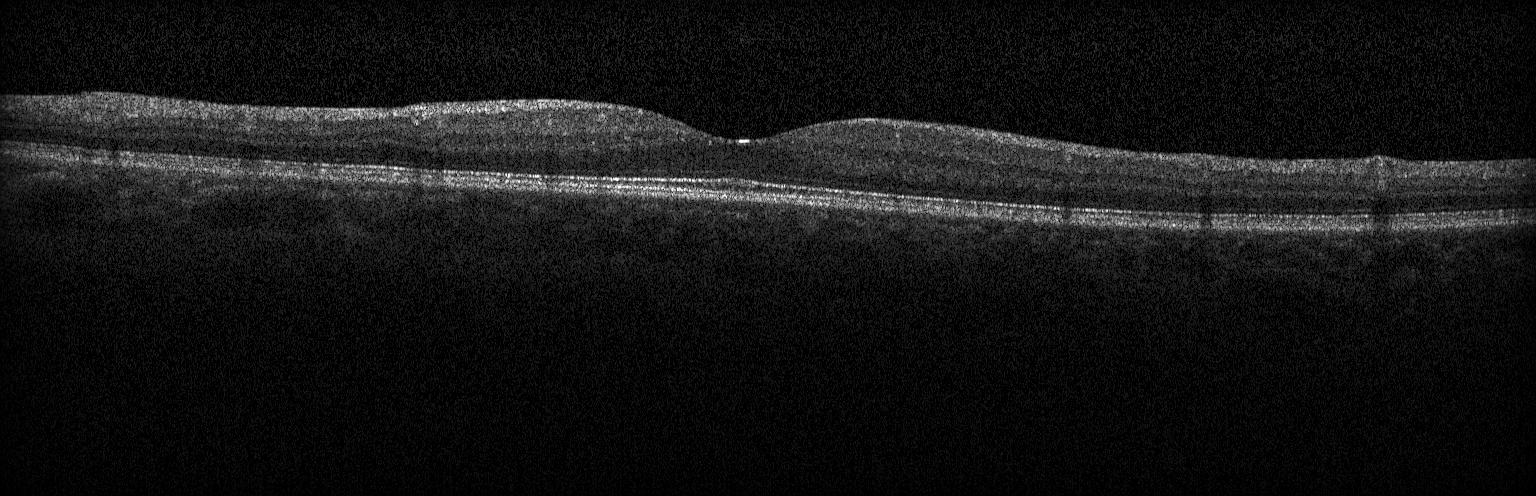 Macular OCT: no choroidal neovascularization, diabetic macular edema, or drusen.